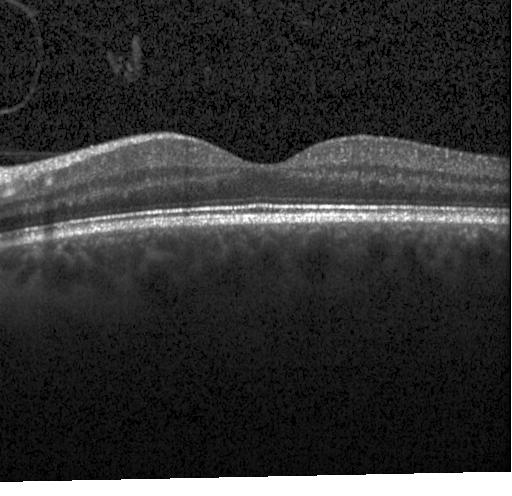 Retinal OCT cross-section
OCT finding: no evidence of CNV, DME, or drusen.